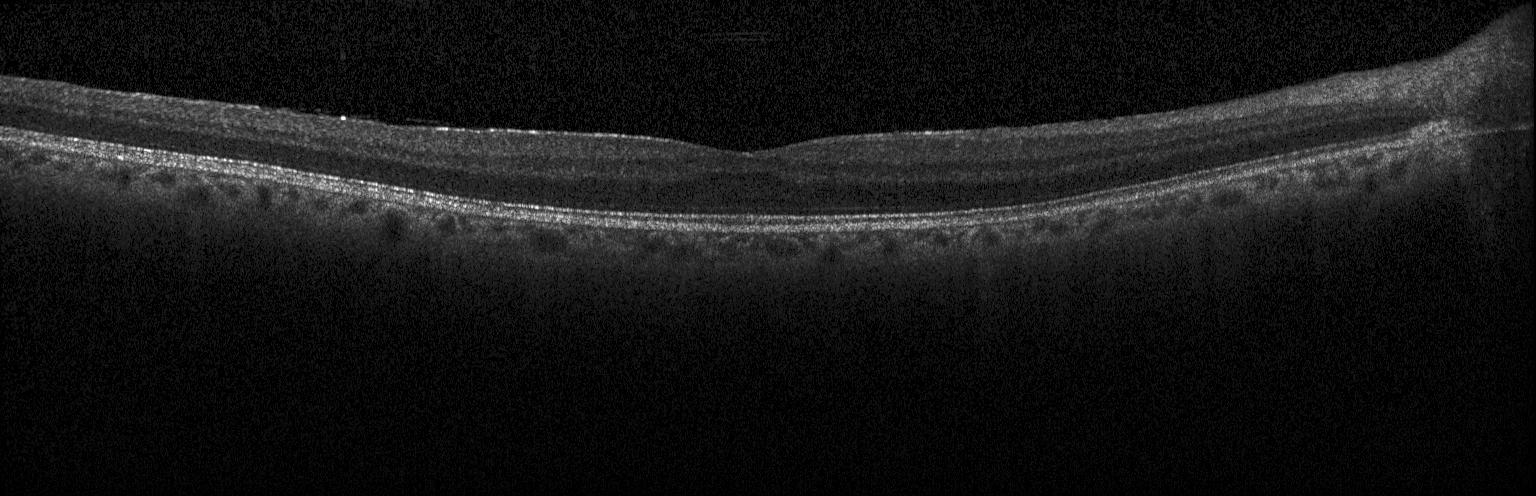
OCT finding: no choroidal neovascularization, diabetic macular edema, or drusen.